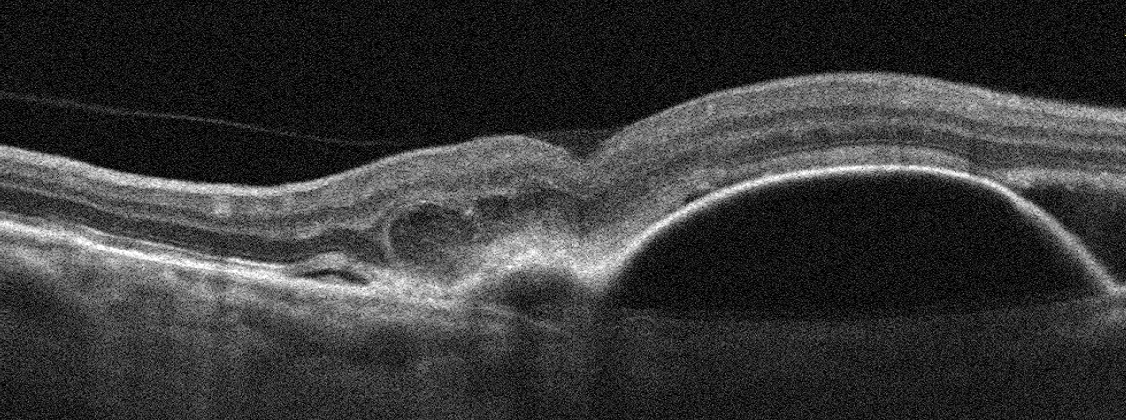

Retinal OCT cross-section; through the macula
This B-scan demonstrates age-related macular degeneration.